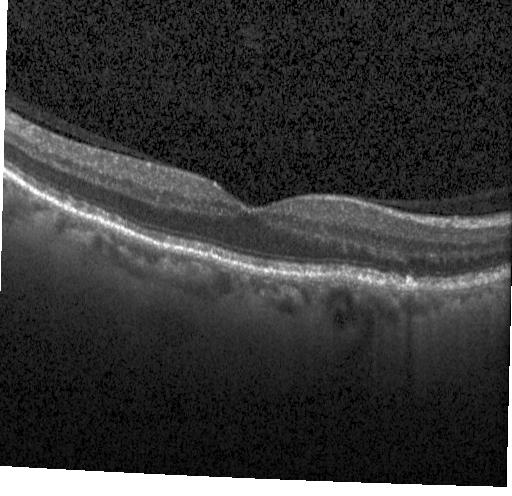
Centered on the fovea; spectral-domain optical coherence tomography; OCT B-scan; acquired on a Heidelberg Spectralis
This B-scan demonstrates no choroidal neovascularization, no diabetic macular edema, and no drusen.